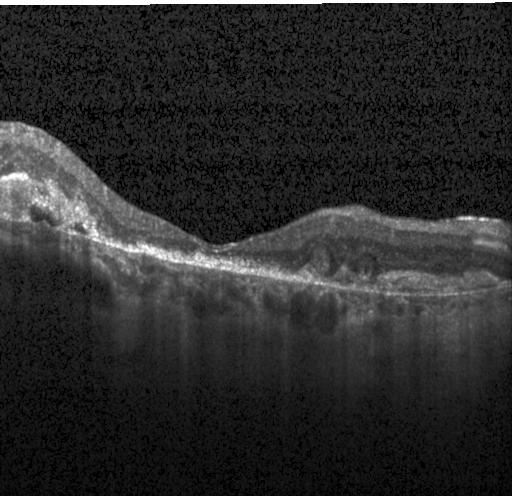
Heidelberg Spectralis · centered on the fovea · OCT line scan.
Impression: a choroidal neovascular membrane.